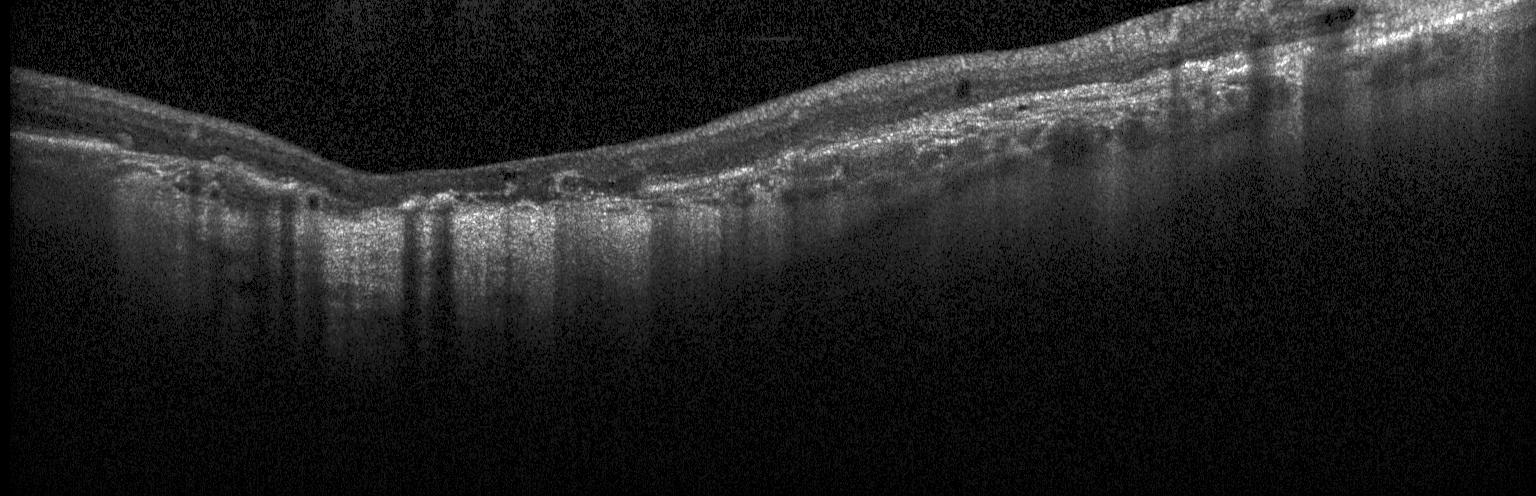
Through the macula; SD-OCT; OCT B-scan.
Assessment: a choroidal neovascular membrane.